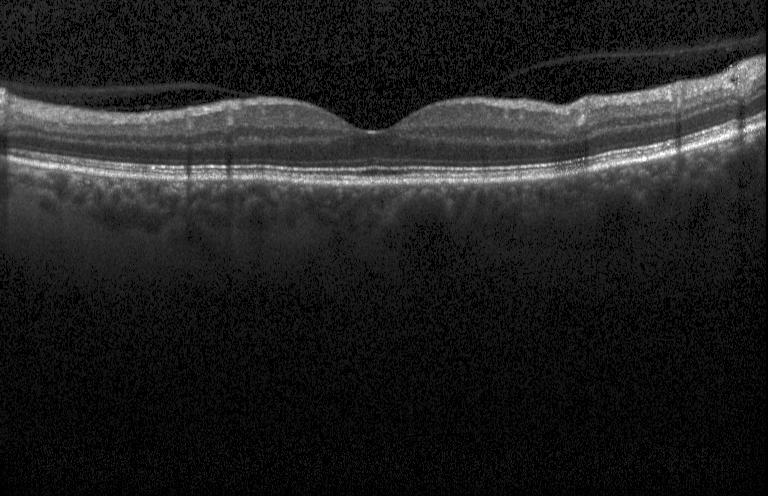 Spectral-domain OCT B-scan: neither choroidal neovascularization, diabetic macular edema, nor drusen.